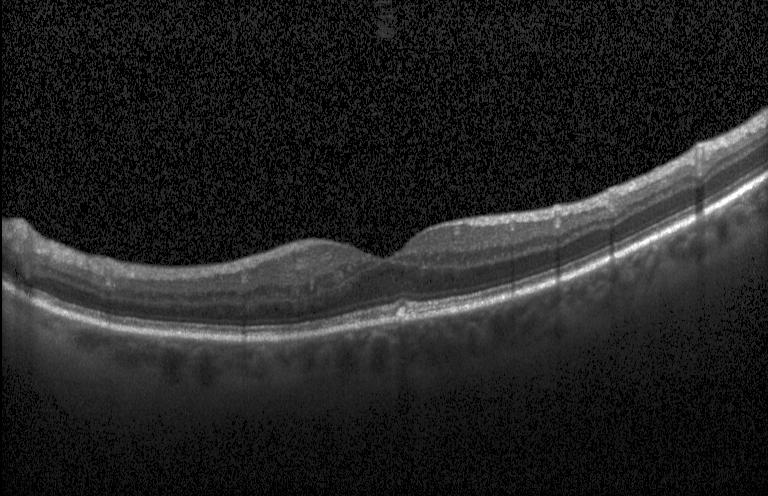 Retinal OCT B-scan — Finding: neither choroidal neovascularization, diabetic macular edema, nor drusen.